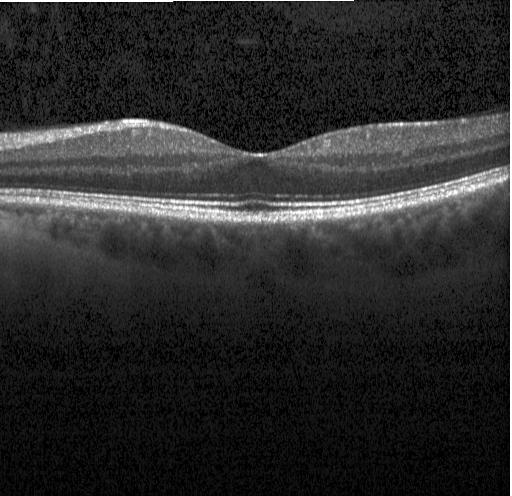 OCT line scan; macular scan — Finding: no choroidal neovascularization, no diabetic macular edema, and no drusen.